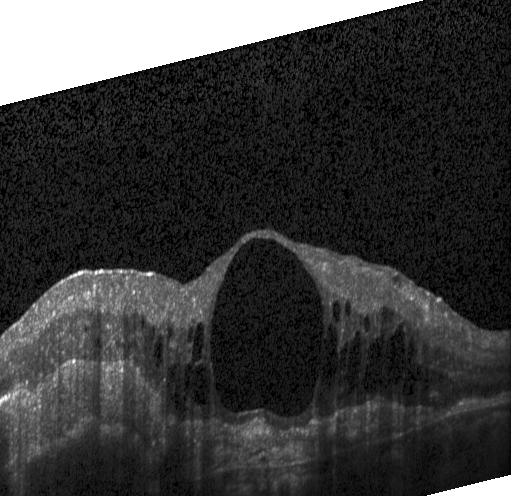 A choroidal neovascular membrane.